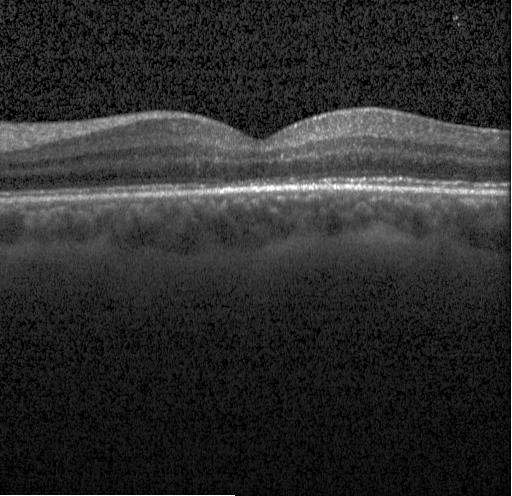
OCT B-scan. Instrument: Heidelberg Spectralis. Centered on the fovea. Spectral-domain OCT — Impression: no CNV, DME, or drusen.